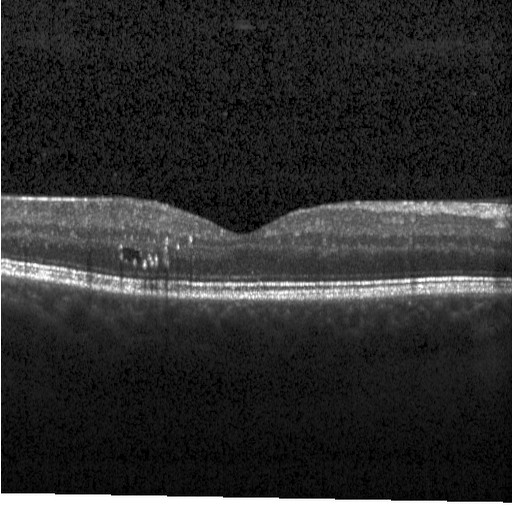
Impression: diabetic macular edema.